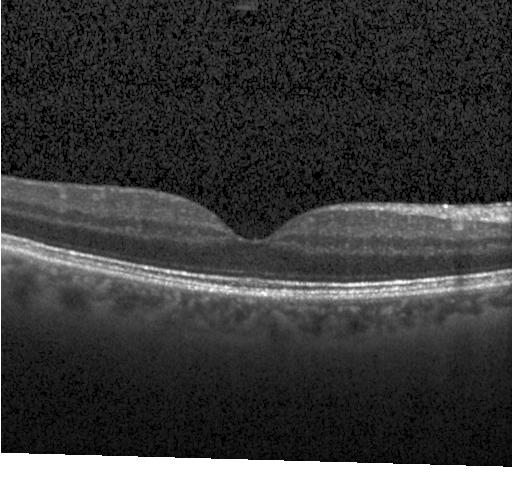
Retinal OCT B-scan.
Impression: no evidence of choroidal neovascularization, diabetic macular edema, or drusen.